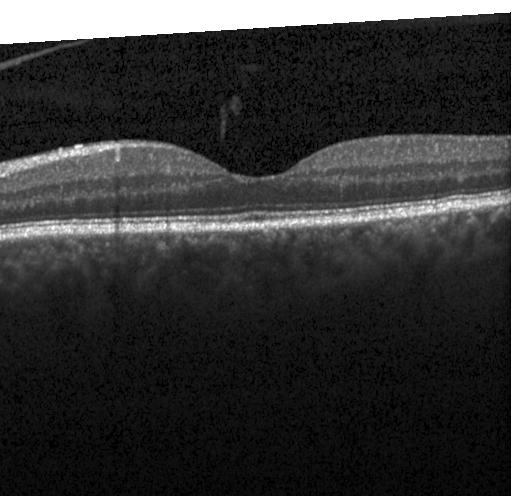 Finding: neither choroidal neovascularization, diabetic macular edema, nor drusen.